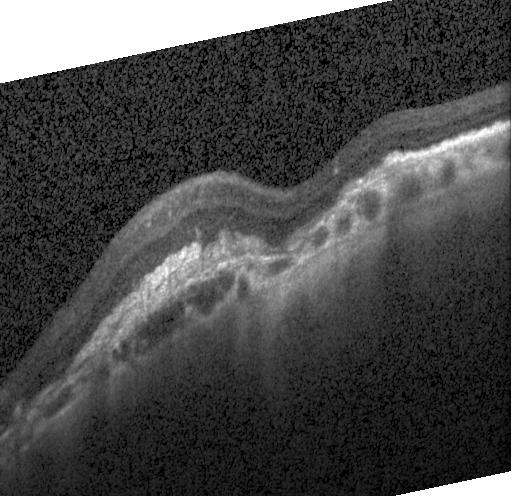

Centered on the fovea. SD-OCT. Acquired on a Heidelberg Spectralis. Retinal OCT B-scan — Dx: a choroidal neovascular membrane.